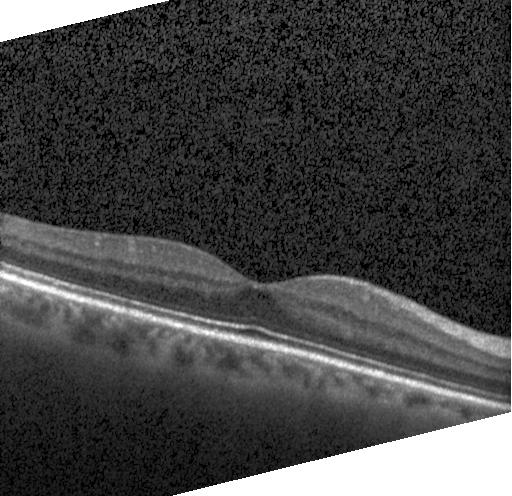 Spectral-domain optical coherence tomography; optical coherence tomography scan; macular scan; acquired on a Heidelberg Spectralis.
No choroidal neovascularization, diabetic macular edema, or drusen.